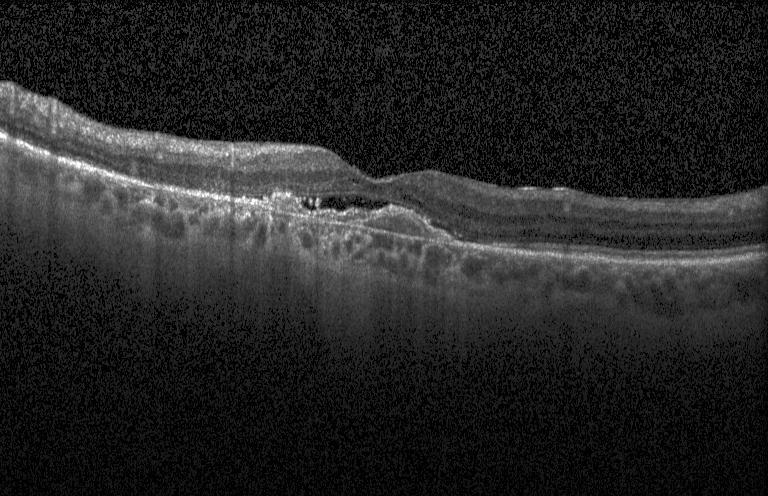 Horizontal scan through the fovea, acquired on a Heidelberg Spectralis, retinal OCT B-scan — A choroidal neovascular membrane.